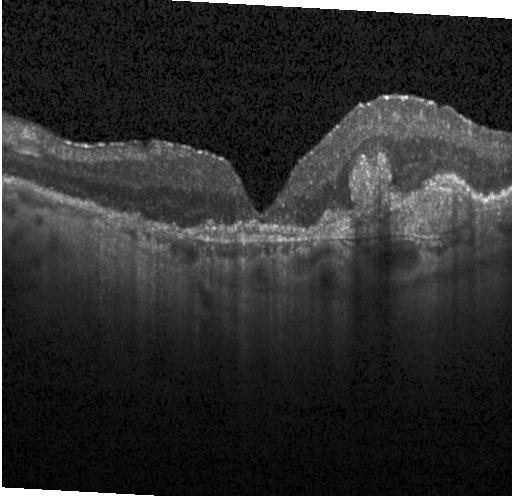
Diagnosis: choroidal neovascularization (CNV).